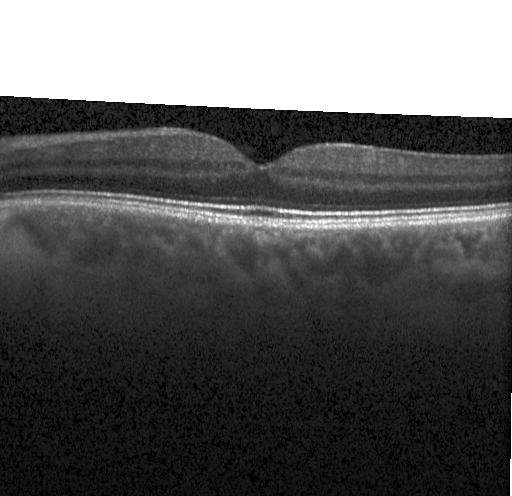
Heidelberg Spectralis OCT system; OCT line scan
The scan shows no choroidal neovascularization, no diabetic macular edema, and no drusen.